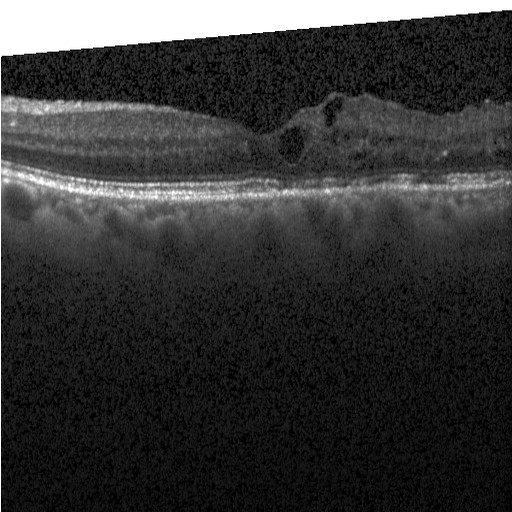

Retinal OCT cross-section showing DME.